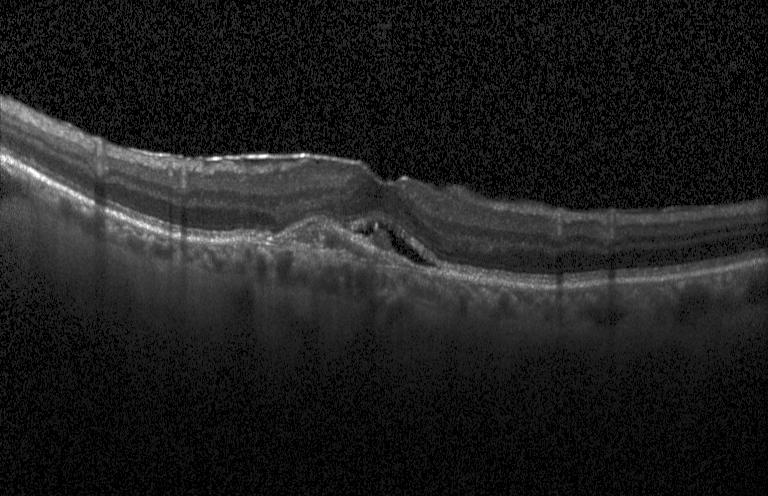
Optical coherence tomography scan; SD-OCT.
Finding: choroidal neovascularization.